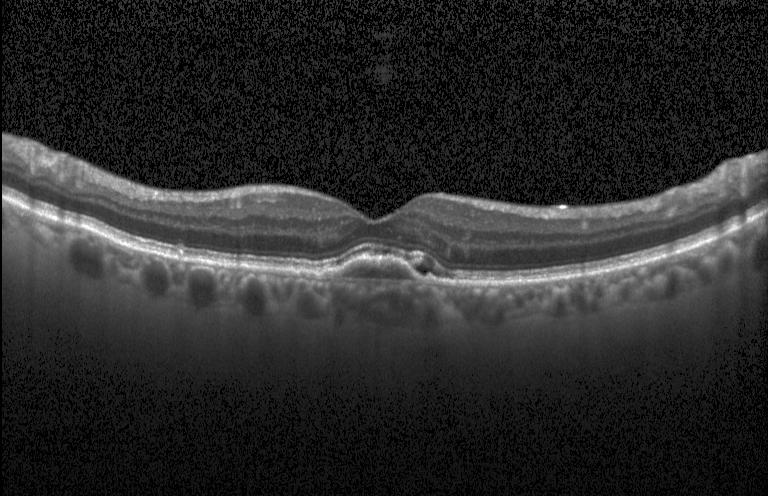

OCT B-scan. Heidelberg Spectralis. Fovea-centered. A choroidal neovascular membrane.